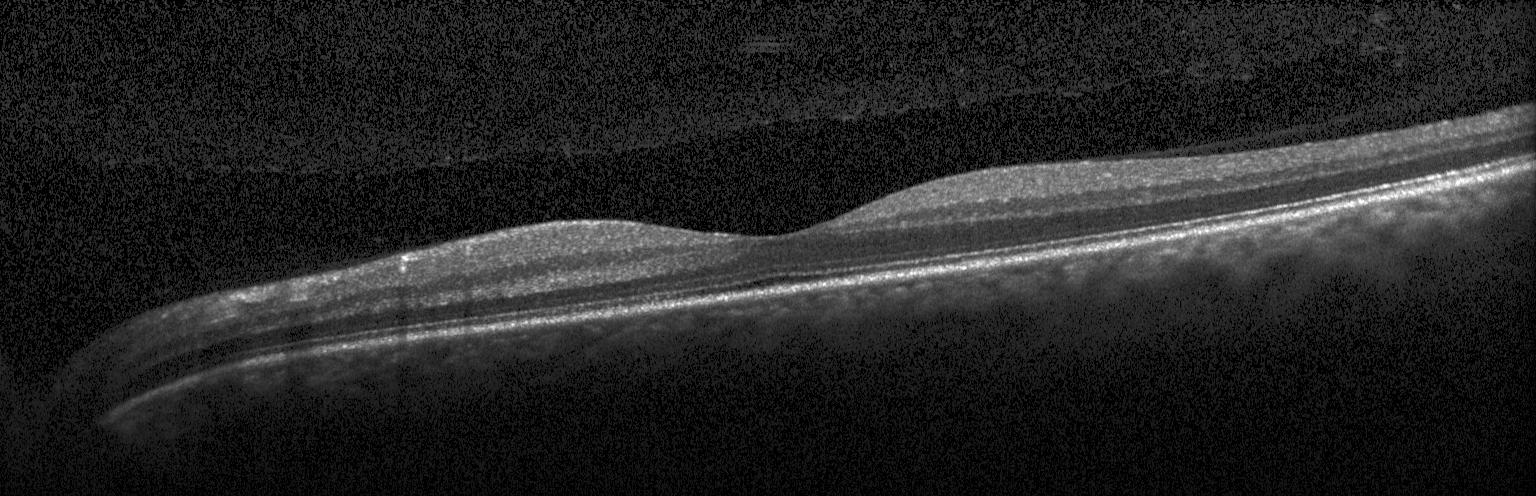

Impression: no choroidal neovascularization, diabetic macular edema, or drusen.